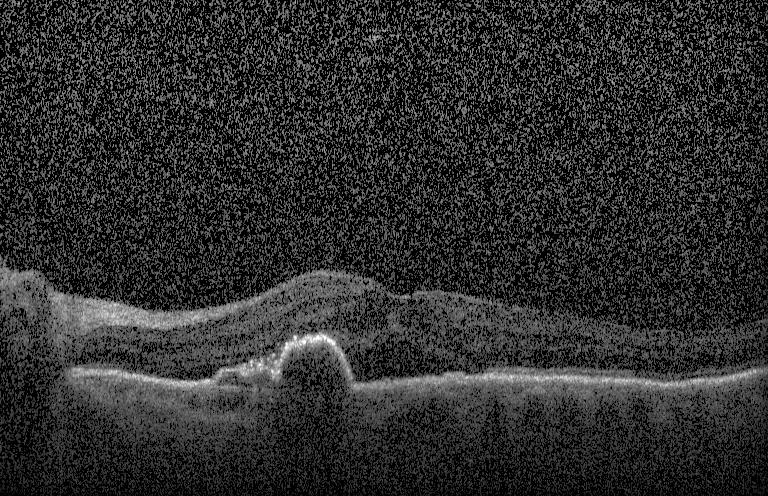 Retinal OCT cross-section. Macular OCT: choroidal neovascularization (CNV).